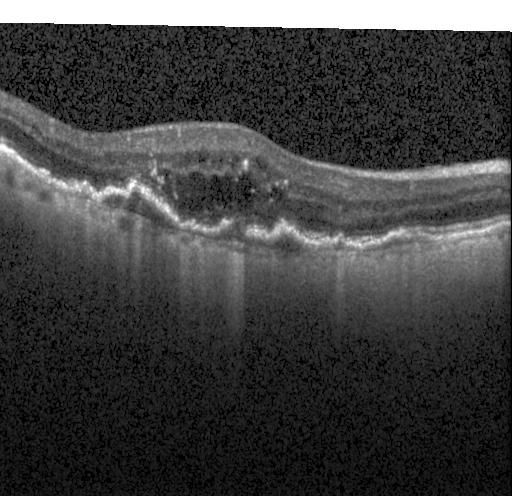

Spectral-domain OCT · centered on the fovea · optical coherence tomography scan · Heidelberg Spectralis — Impression: a choroidal neovascular membrane.